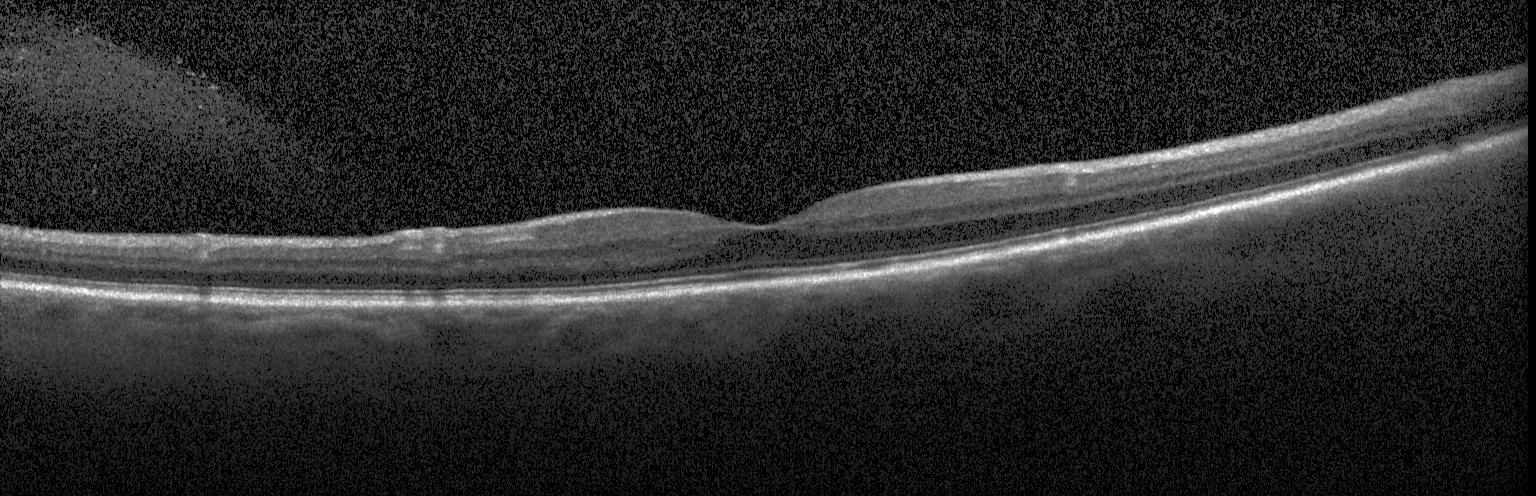
OCT B-scan. Acquired on a Heidelberg Spectralis. Dx: no CNV, DME, or drusen.